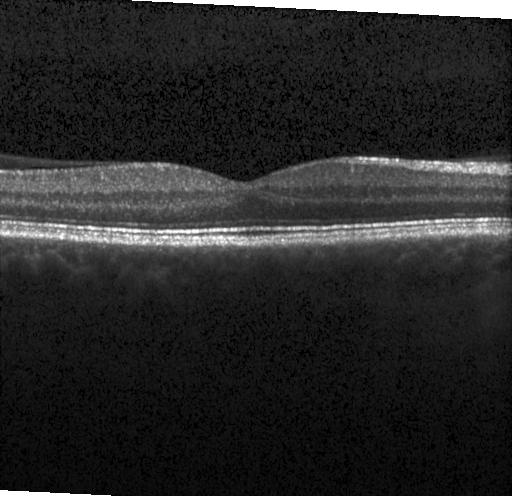 Diagnosis: no CNV, no DME, and no drusen.